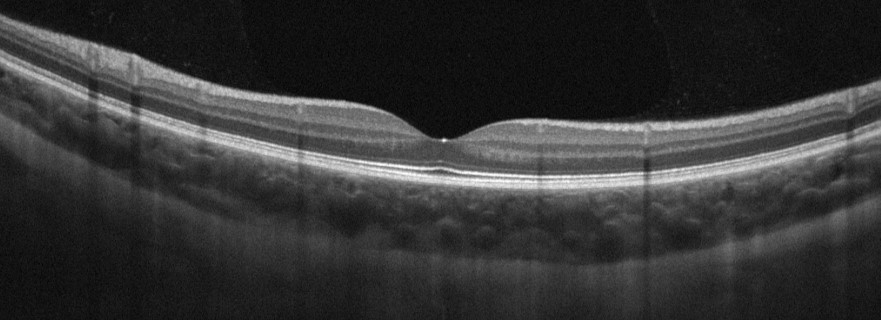 OCT finding: no AMD, DME, ERM, RAO, RVO, or VID.